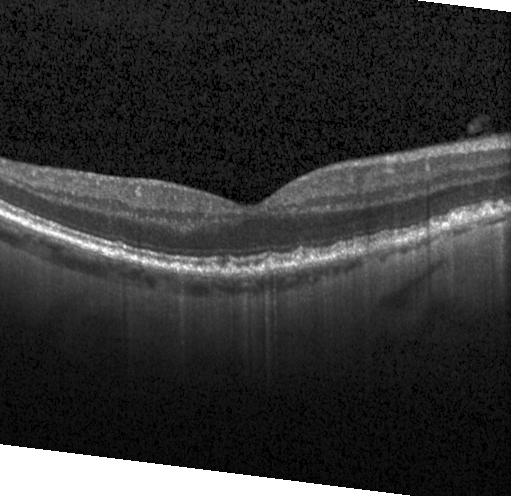

OCT line scan.
Impression: sub-RPE drusenoid deposits.